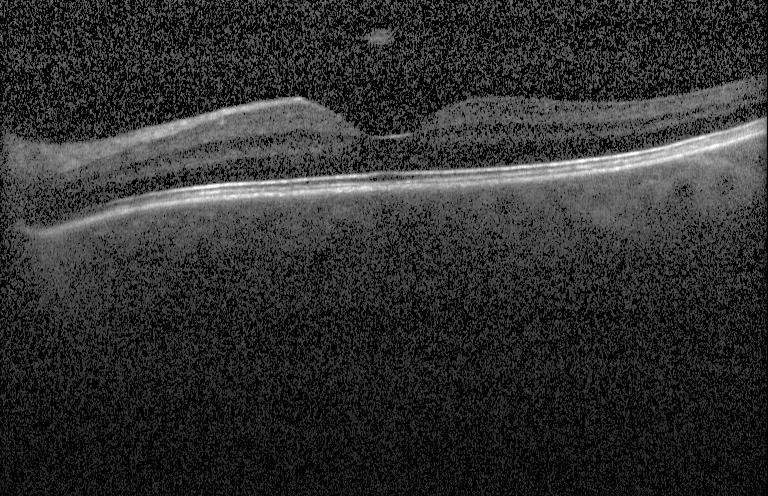

Through the macula, Heidelberg Spectralis, retinal OCT B-scan. Assessment: no choroidal neovascularization, diabetic macular edema, or drusen.